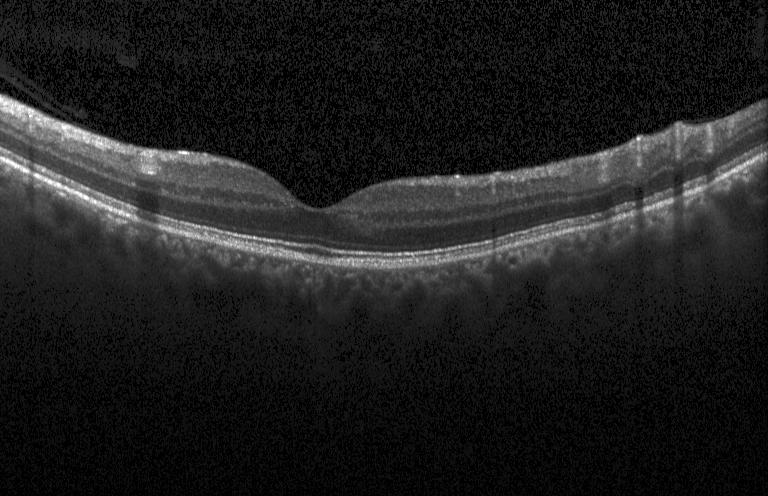 SD-OCT · retinal OCT B-scan · Heidelberg Spectralis OCT system. Diagnosis: no CNV, no DME, and no drusen.